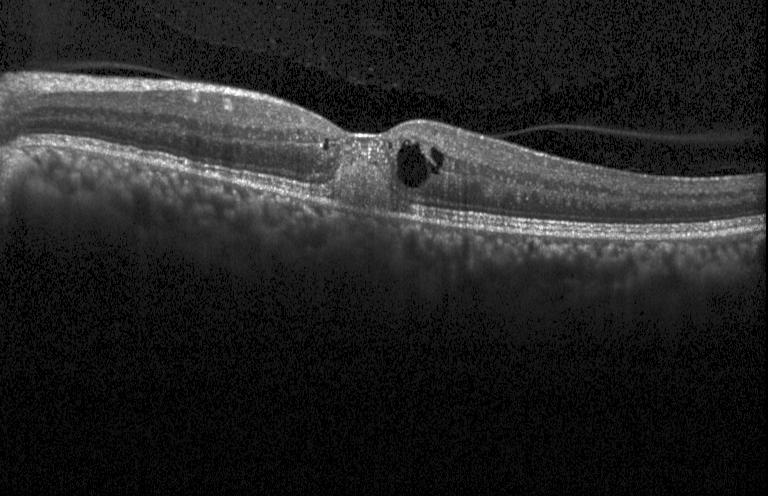 Heidelberg Spectralis OCT system · retinal OCT cross-section · through the macula · spectral-domain optical coherence tomography.
Dx: a choroidal neovascular membrane.